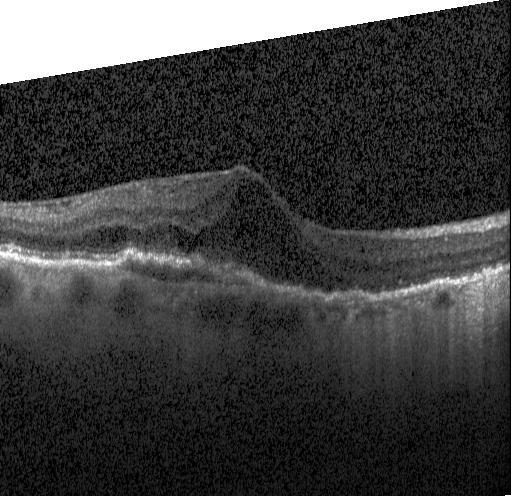

Dx: a choroidal neovascular membrane.